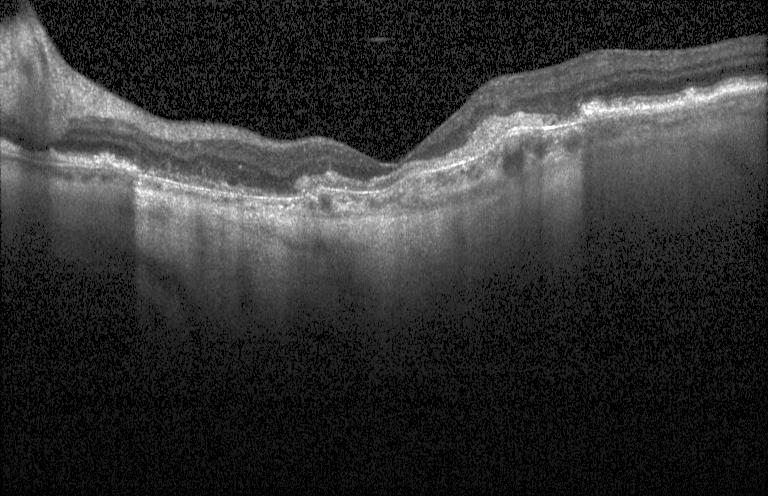
SD-OCT; fovea-centered; retinal OCT B-scan — Dx: CNV.